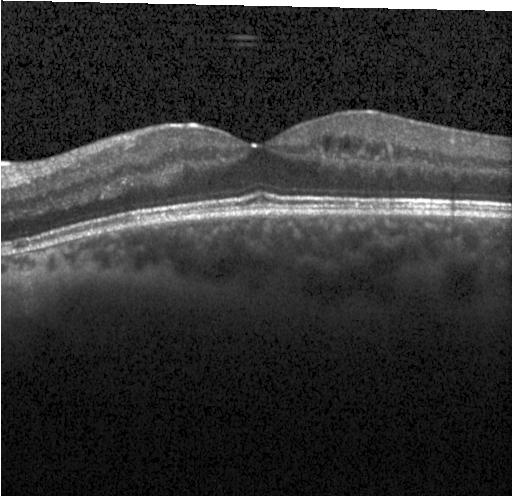
Retinal OCT B-scan
The scan shows DME.